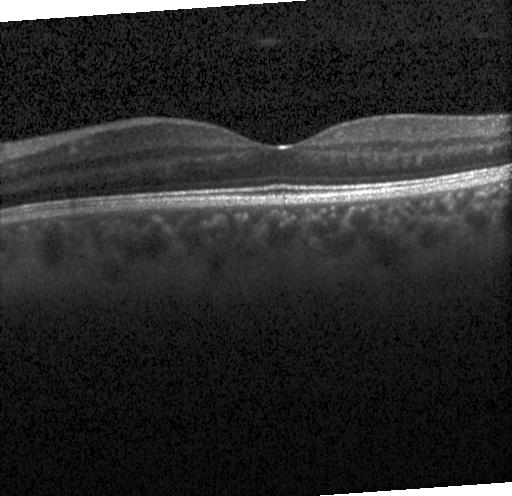

Spectral-domain optical coherence tomography; macular scan; OCT B-scan; instrument: Heidelberg Spectralis — Diagnosis: neither CNV, DME, nor drusen.